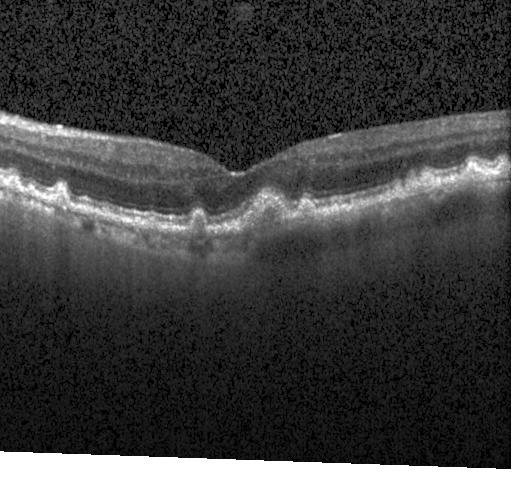

Retinal OCT B-scan, Heidelberg Spectralis, spectral-domain OCT, fovea-centered.
Diagnosis: drusen.